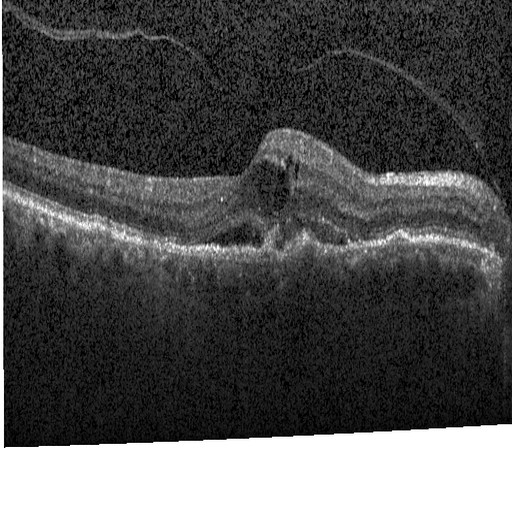
OCT B-scan showing diabetic macular edema (DME).